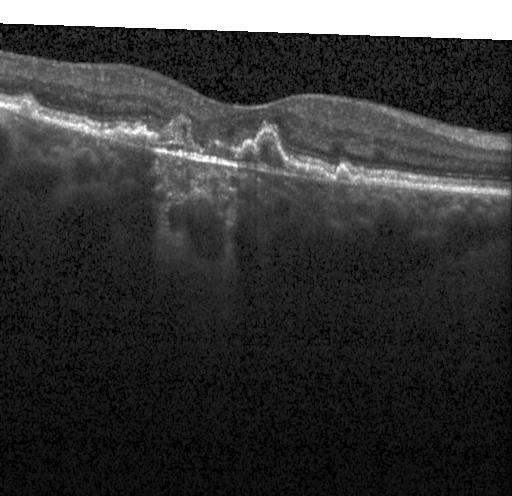
CNV.